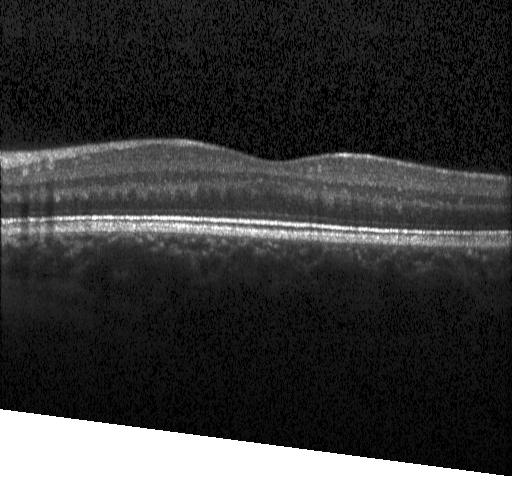
Finding: no choroidal neovascularization, no diabetic macular edema, and no drusen.